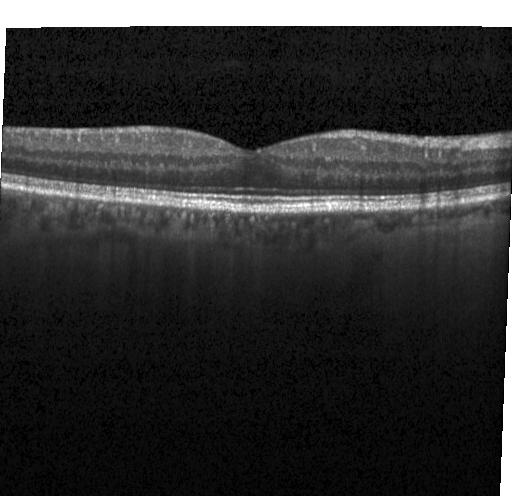 Spectral-domain OCT · optical coherence tomography B-scan · instrument: Heidelberg Spectralis · through the macula
OCT finding: no CNV, no DME, and no drusen.